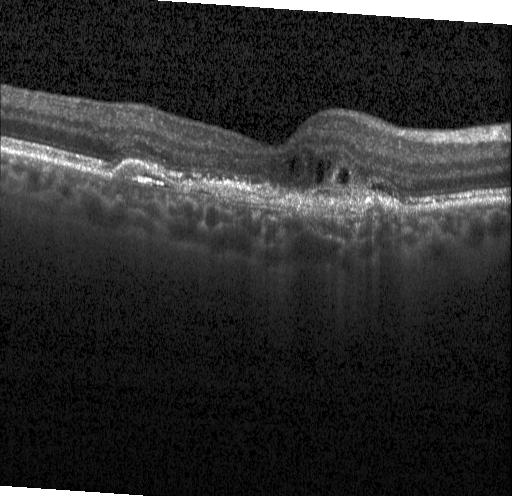 Centered on the fovea; Heidelberg Spectralis; OCT line scan
Finding: a choroidal neovascular membrane.